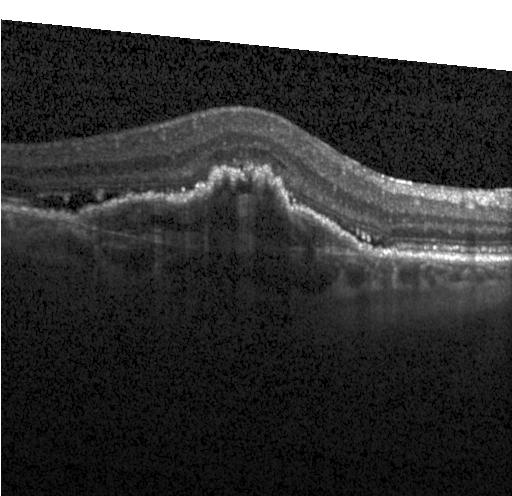

Finding: a choroidal neovascular membrane.